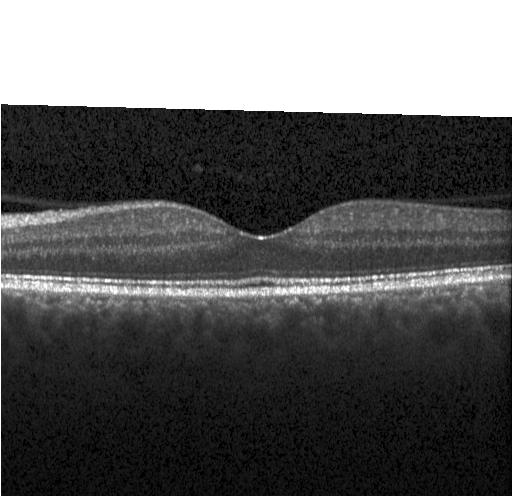
Optical coherence tomography B-scan — Finding: no choroidal neovascularization, diabetic macular edema, or drusen.